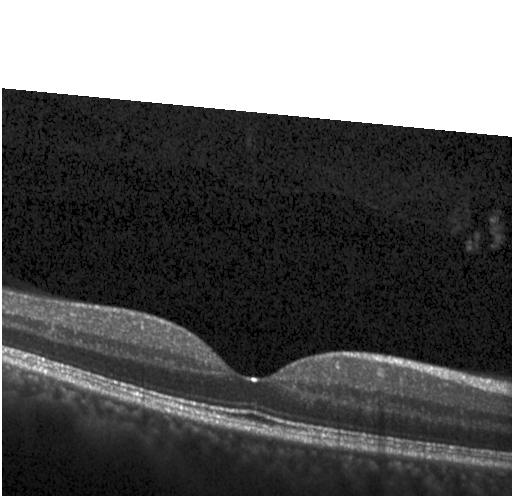

The scan shows neither choroidal neovascularization, diabetic macular edema, nor drusen.